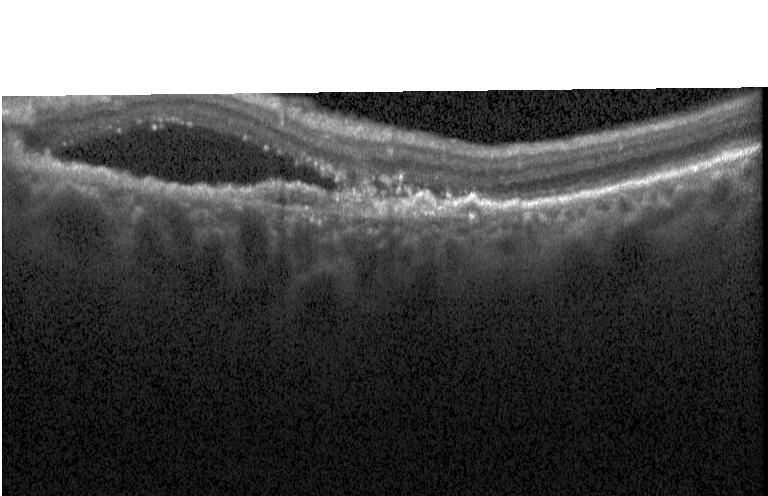 Optical coherence tomography B-scan, spectral-domain optical coherence tomography, Heidelberg Spectralis — Diagnosis: a choroidal neovascular membrane.